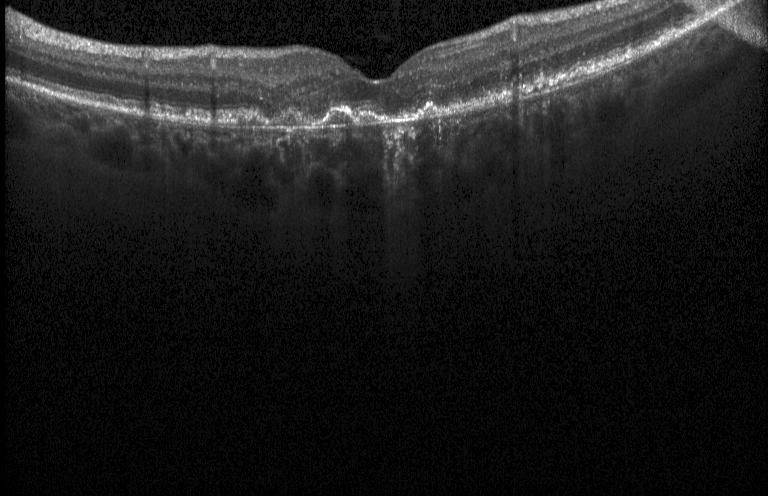
Macular OCT demonstrating a choroidal neovascular membrane.